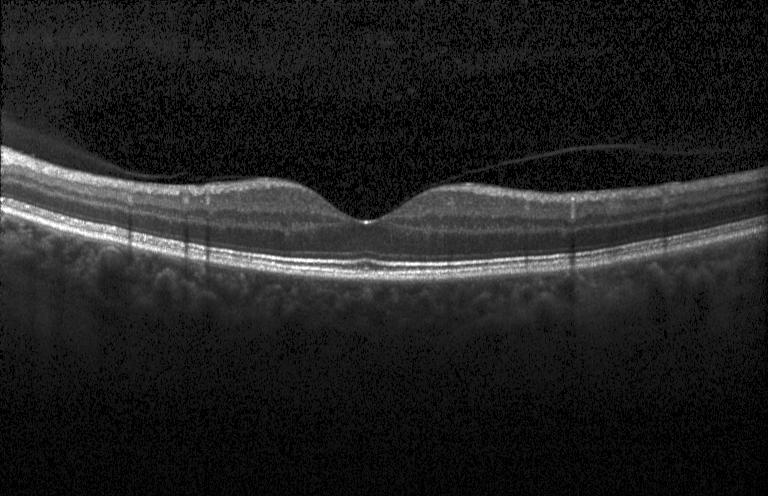
Through the macula; OCT line scan; spectral-domain OCT — Macular OCT: no evidence of choroidal neovascularization, diabetic macular edema, or drusen.